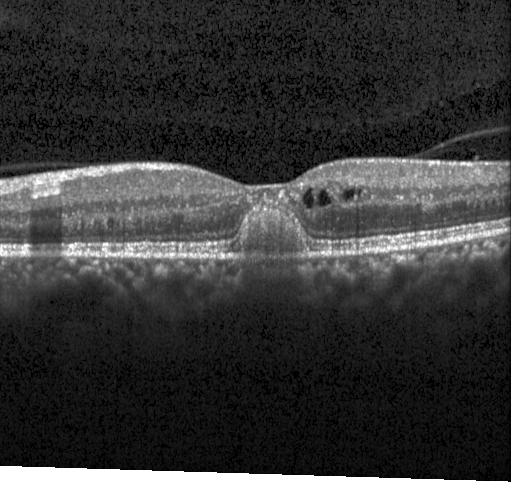 Spectral-domain OCT; optical coherence tomography B-scan — Macular OCT: a choroidal neovascular membrane.